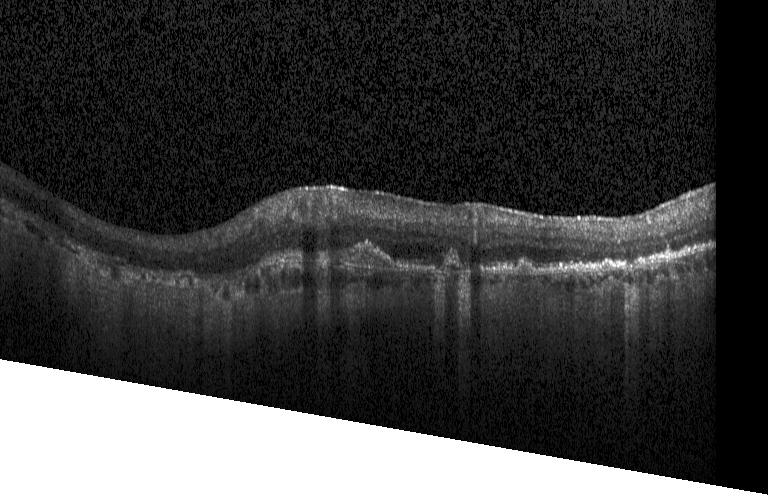
OCT line scan · acquired on a Heidelberg Spectralis · spectral-domain optical coherence tomography — Choroidal neovascularization.